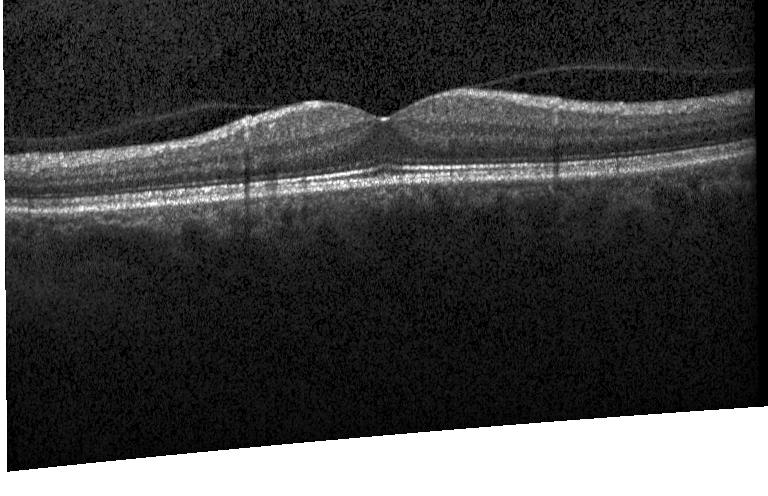

Spectral-domain OCT; fovea-centered; instrument: Heidelberg Spectralis; OCT B-scan. No evidence of choroidal neovascularization, diabetic macular edema, or drusen.